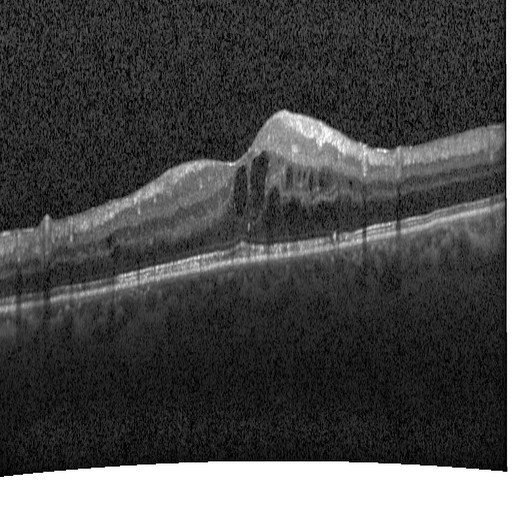
Optical coherence tomography scan — Impression: diabetic macular edema.